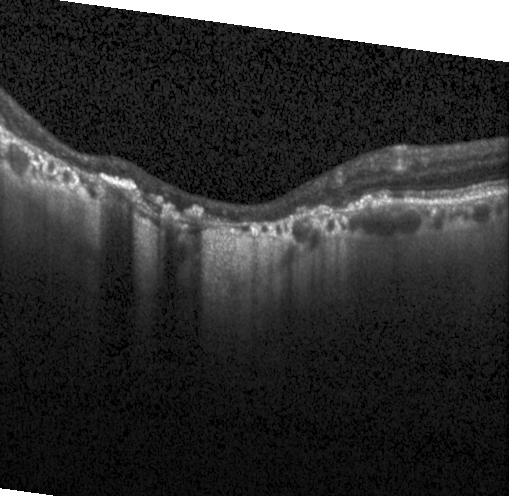
Spectral-domain OCT B-scan: a choroidal neovascular membrane.